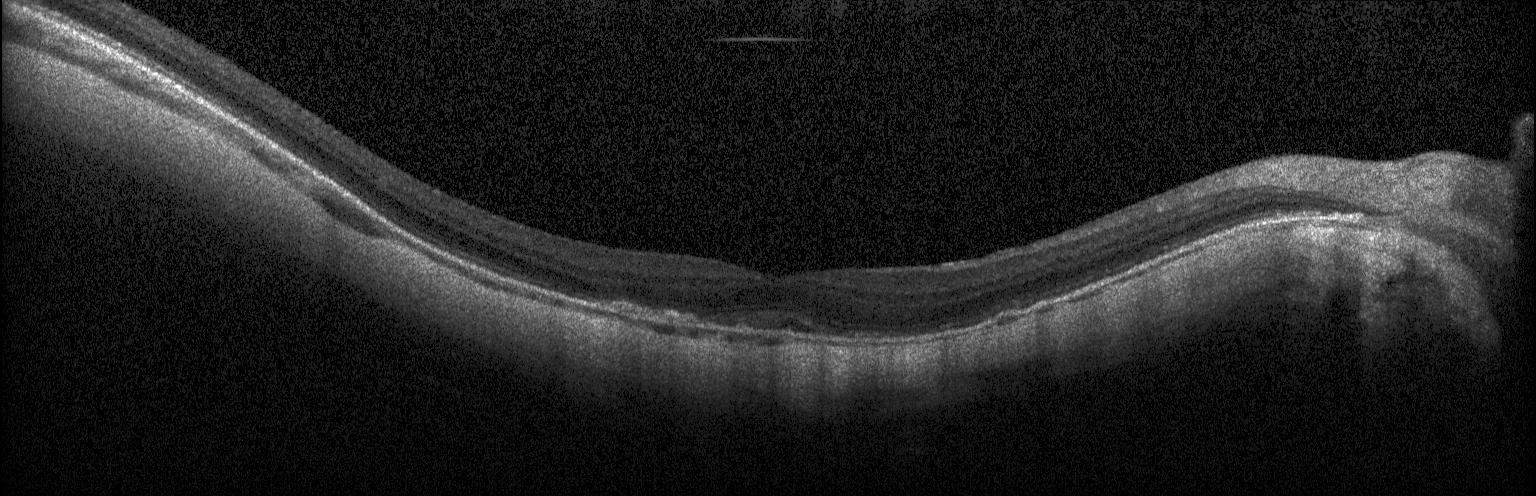
CNV.